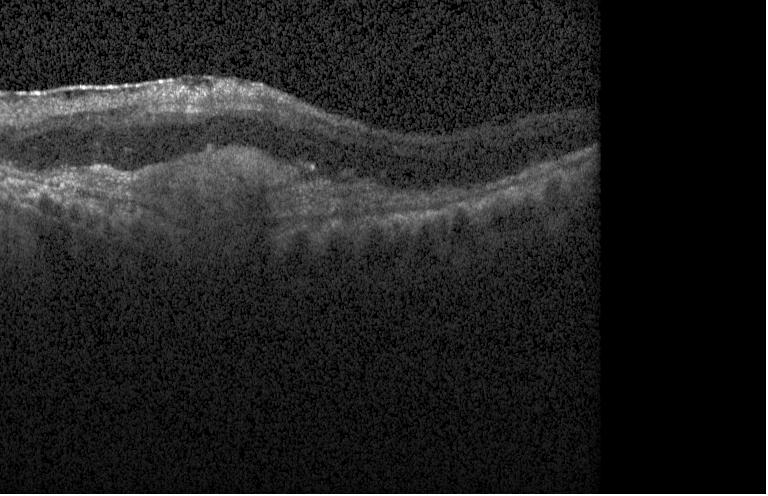 Optical coherence tomography B-scan, SD-OCT, Heidelberg Spectralis OCT system — OCT finding: CNV.